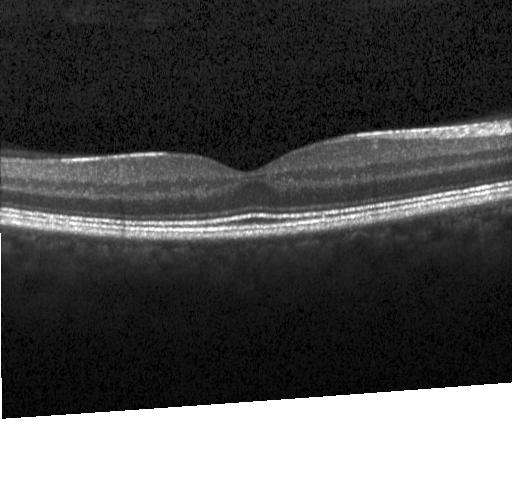
OCT finding: no CNV, no DME, and no drusen.